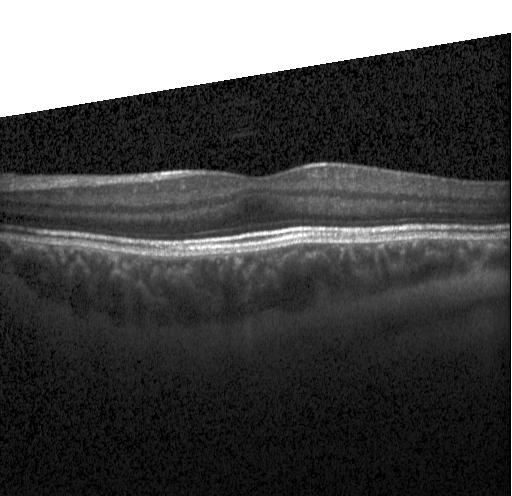 OCT B-scan showing neither choroidal neovascularization, diabetic macular edema, nor drusen.